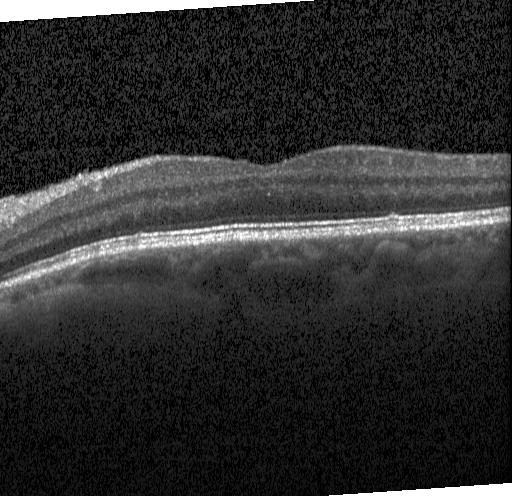 Retinal OCT cross-section
Macular OCT: no choroidal neovascularization, no diabetic macular edema, and no drusen.